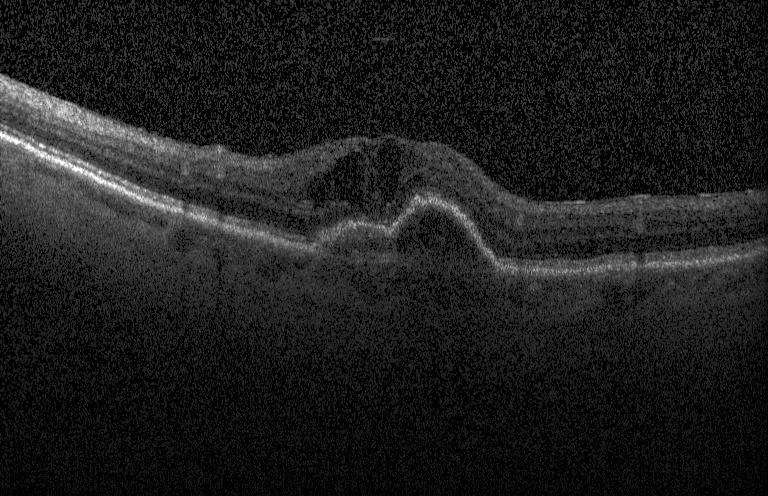

Retinal OCT B-scan · acquired on a Heidelberg Spectralis. Impression: choroidal neovascularization.